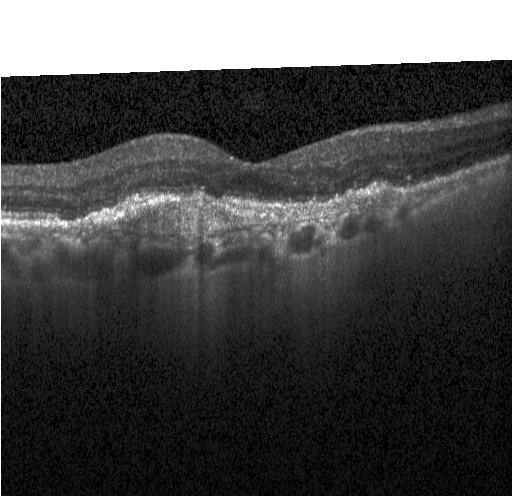
Spectral-domain OCT B-scan: a choroidal neovascular membrane.